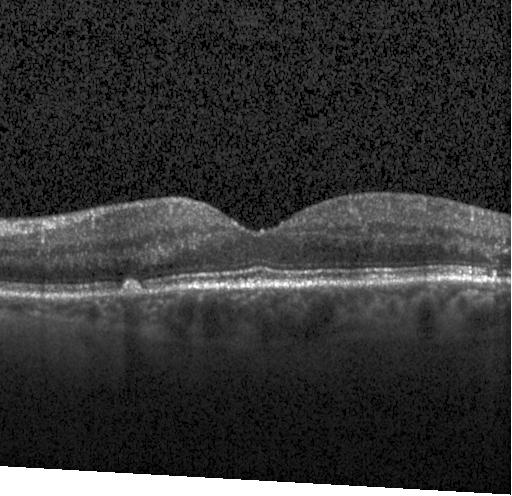 OCT line scan. Macular scan — OCT finding: multiple drusen.